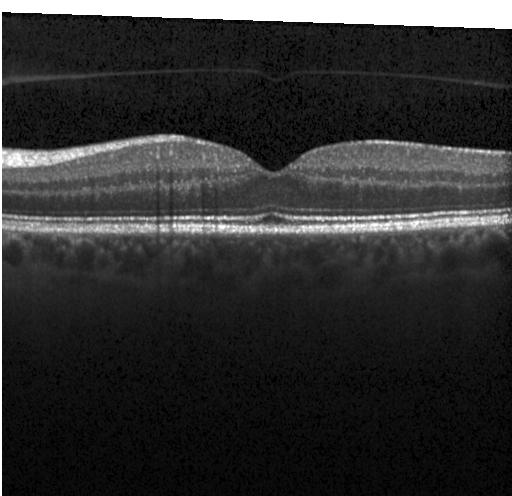

OCT line scan · horizontal scan through the fovea. Finding: neither choroidal neovascularization, diabetic macular edema, nor drusen.